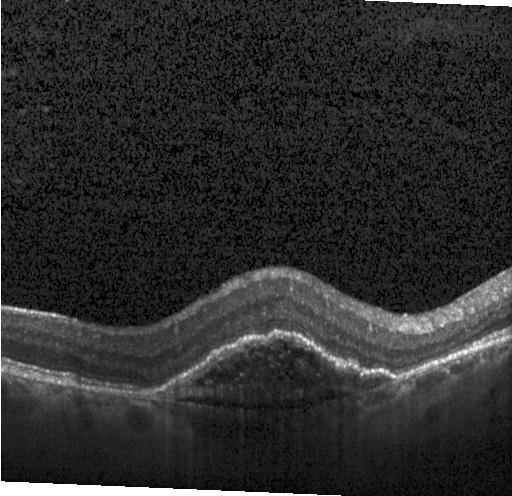
Fovea-centered. Heidelberg Spectralis OCT system. Spectral-domain OCT. Retinal OCT cross-section. Diagnosis: CNV.